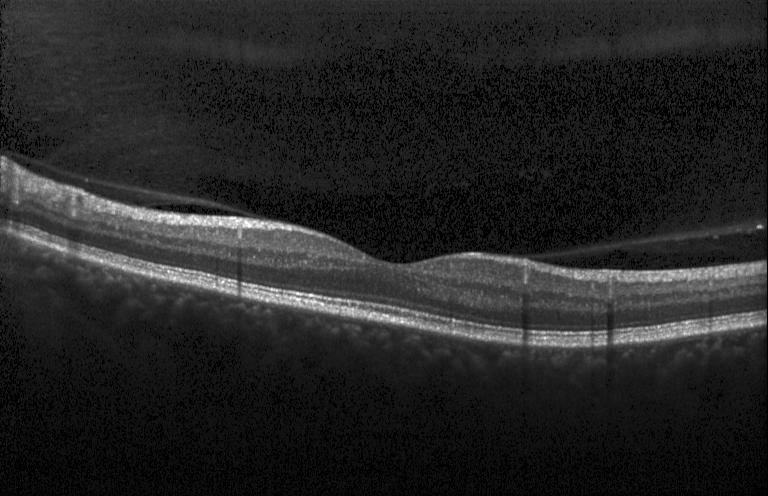 Instrument: Heidelberg Spectralis, retinal OCT B-scan — Impression: neither CNV, DME, nor drusen.